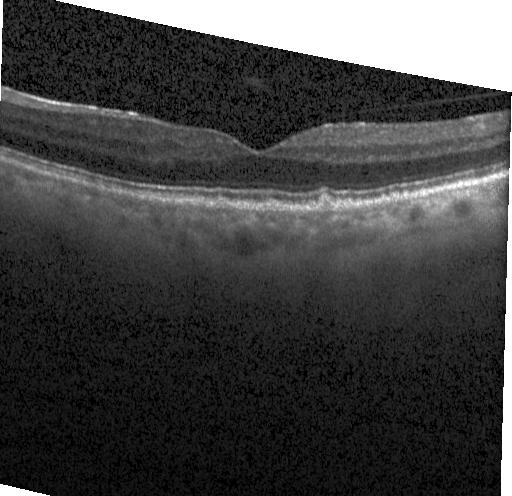

Centered on the fovea, OCT B-scan, spectral-domain optical coherence tomography, Heidelberg Spectralis OCT system.
The scan shows multiple drusen.